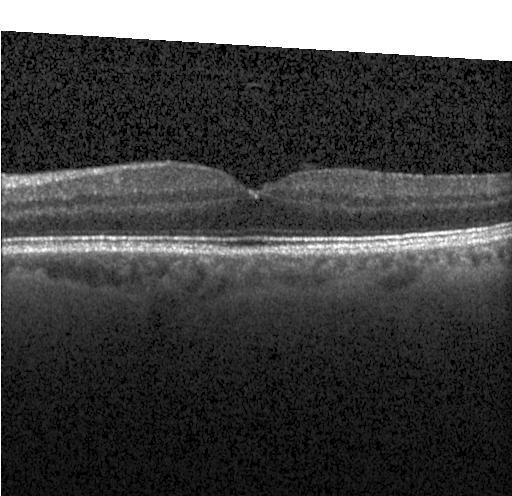 Fovea-centered. OCT line scan — Diagnosis: no choroidal neovascularization, no diabetic macular edema, and no drusen.